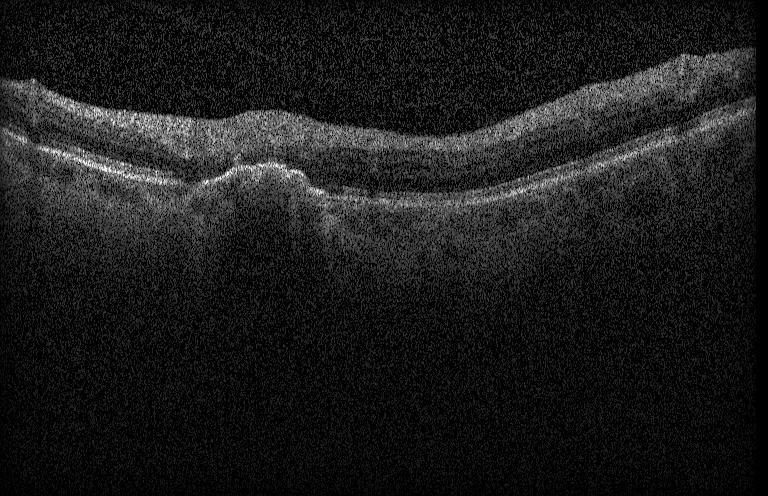 Optical coherence tomography scan. Finding: a choroidal neovascular membrane.